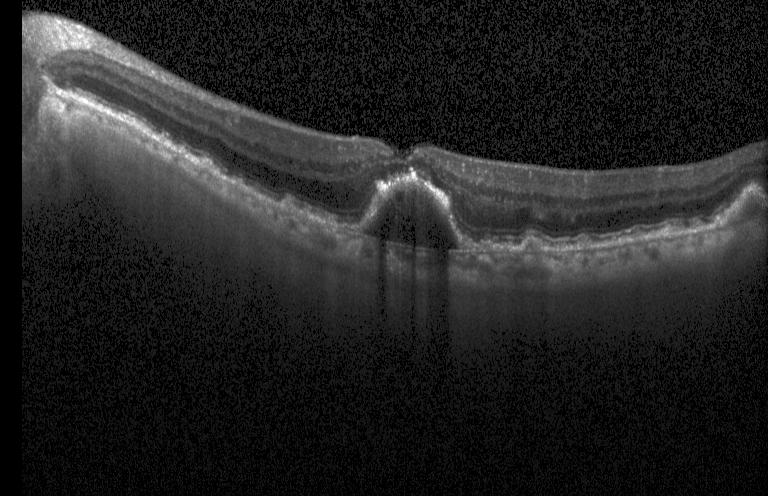
Instrument: Heidelberg Spectralis · SD-OCT · optical coherence tomography B-scan · macular scan. CNV.